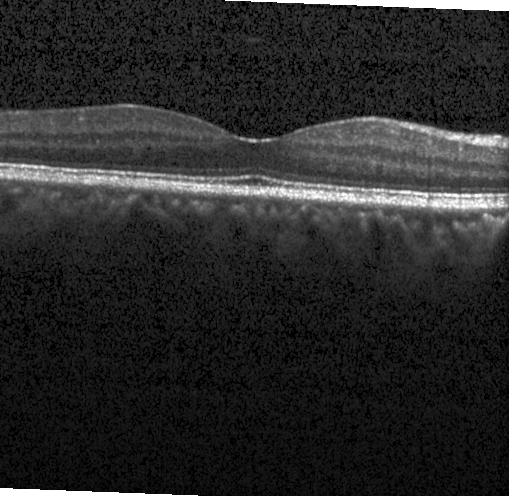

OCT B-scan. Spectral-domain OCT.
Impression: no choroidal neovascularization, no diabetic macular edema, and no drusen.